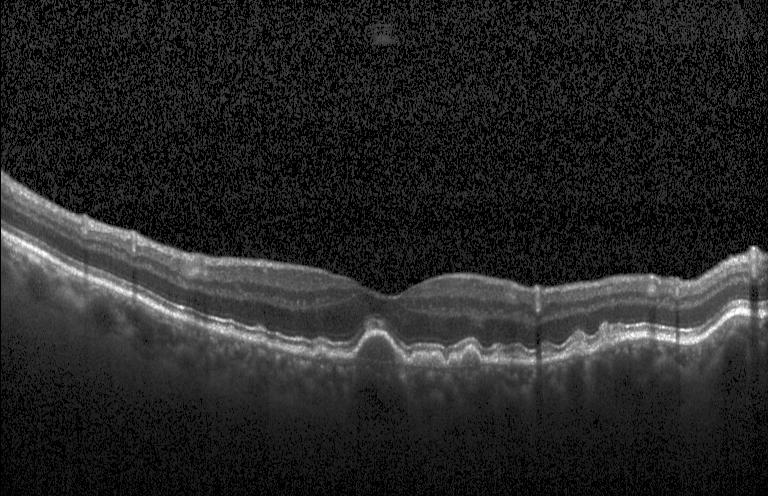

Acquired on a Heidelberg Spectralis, retinal OCT B-scan, SD-OCT — Assessment: sub-RPE drusenoid deposits.